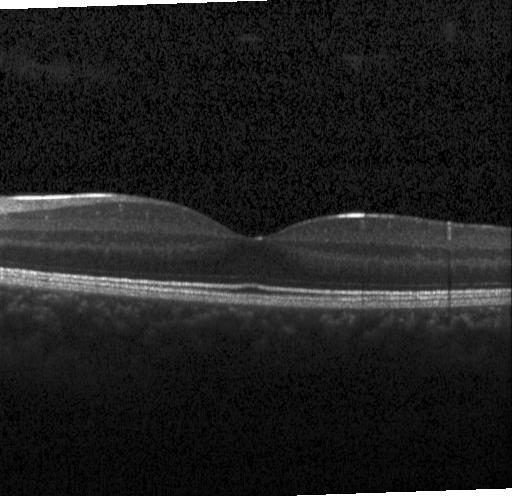

Optical coherence tomography scan — Dx: neither CNV, DME, nor drusen.